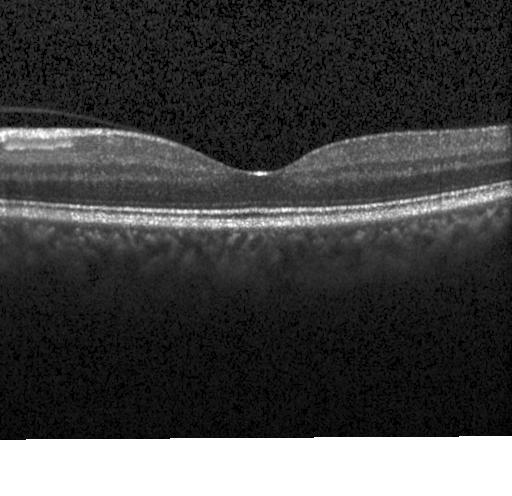

Impression: neither choroidal neovascularization, diabetic macular edema, nor drusen.